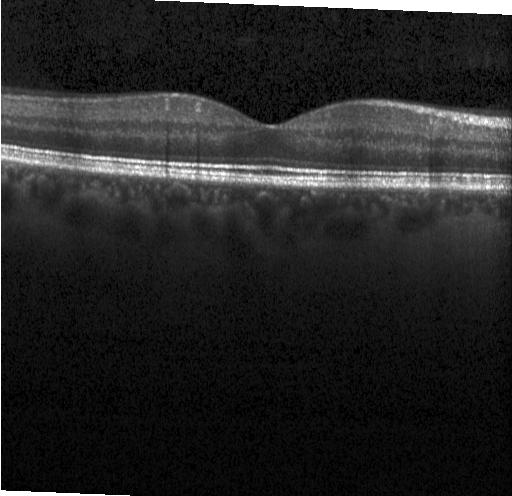 Diagnosis: no CNV, DME, or drusen.